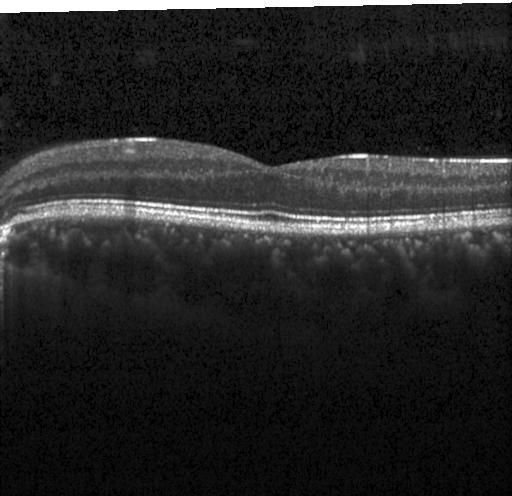

Fovea-centered. OCT line scan. Heidelberg Spectralis. SD-OCT — Macular OCT: neither choroidal neovascularization, diabetic macular edema, nor drusen.